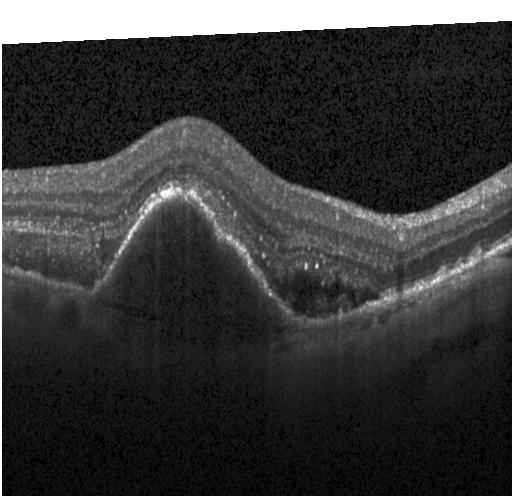 Retinal OCT B-scan
Impression: choroidal neovascularization (CNV).